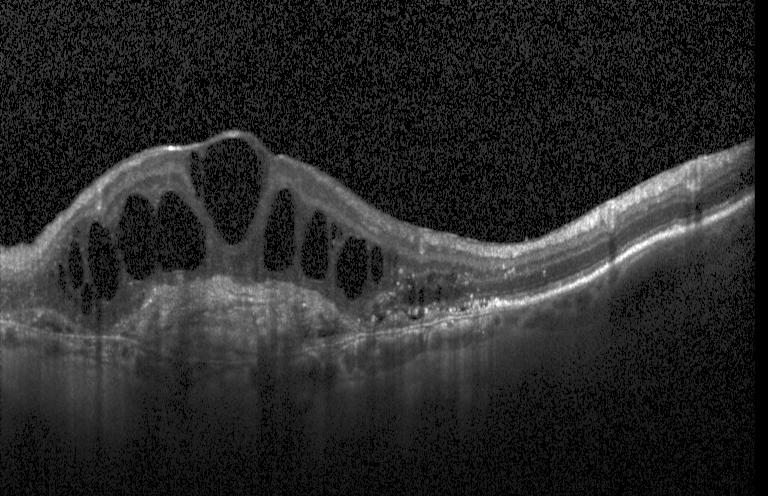
OCT B-scan showing a choroidal neovascular membrane.